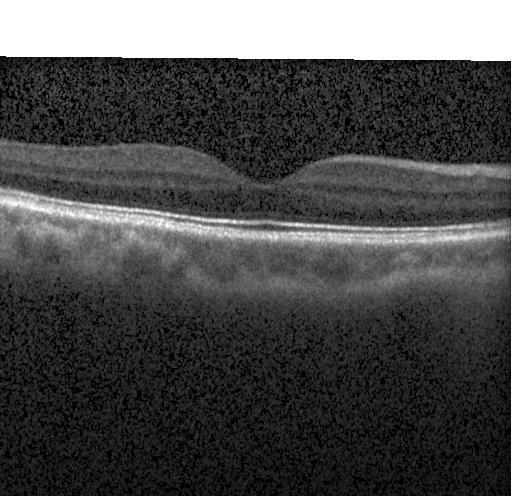
Optical coherence tomography B-scan. Horizontal scan through the fovea. Spectral-domain OCT — Impression: neither CNV, DME, nor drusen.